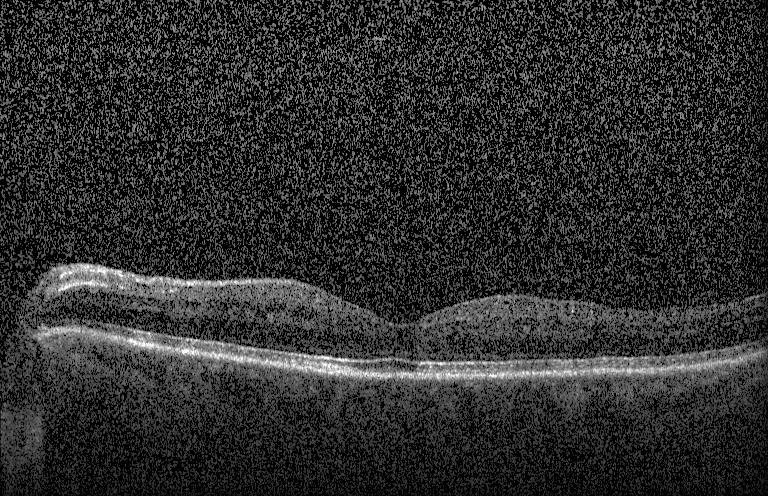

Spectral-domain OCT; instrument: Heidelberg Spectralis; optical coherence tomography B-scan; through the macula. Macular OCT: no CNV, DME, or drusen.